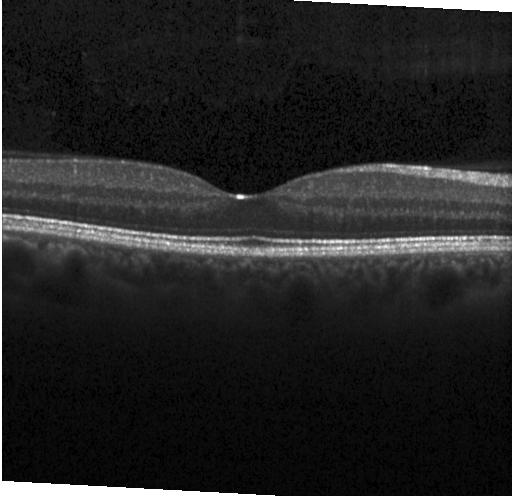
Diagnosis: no evidence of choroidal neovascularization, diabetic macular edema, or drusen.